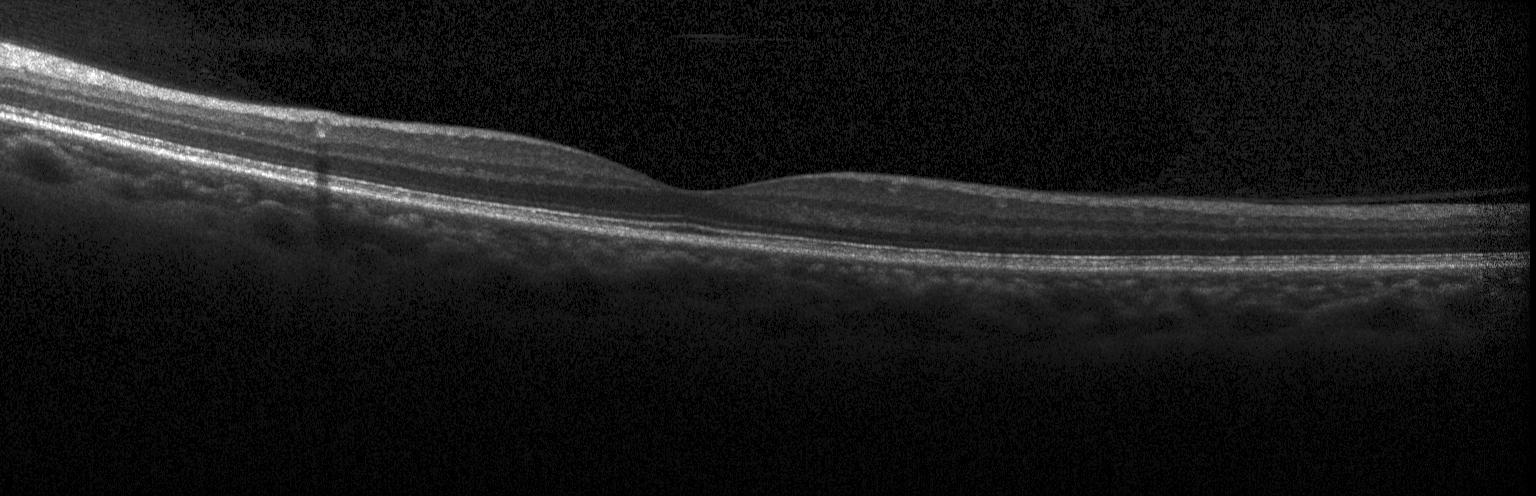
Macular OCT demonstrating no choroidal neovascularization, diabetic macular edema, or drusen.